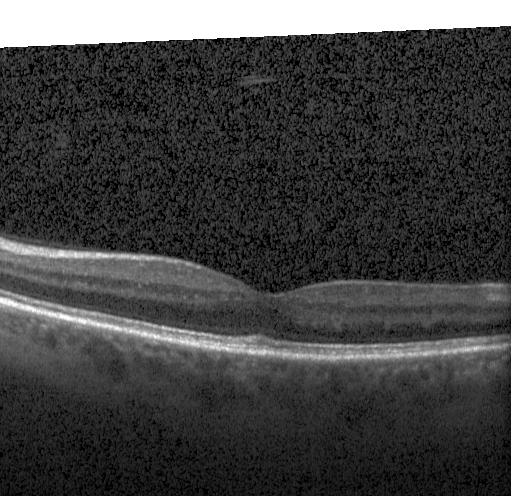 Optical coherence tomography scan, acquired on a Heidelberg Spectralis, SD-OCT — Impression: no evidence of CNV, DME, or drusen.